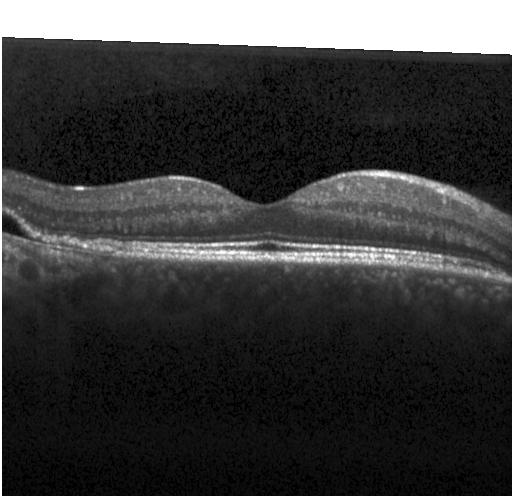
Impression: a choroidal neovascular membrane.